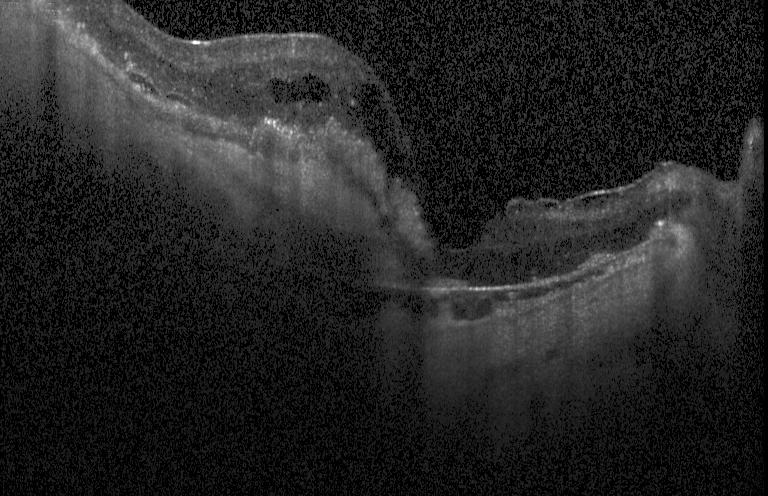
OCT line scan, acquired on a Heidelberg Spectralis
A choroidal neovascular membrane.